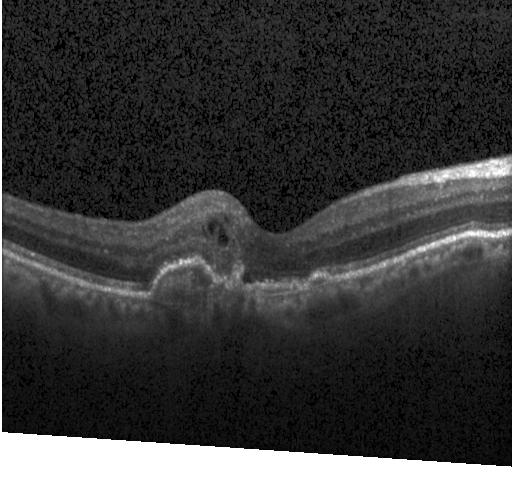 Macular OCT: a choroidal neovascular membrane.